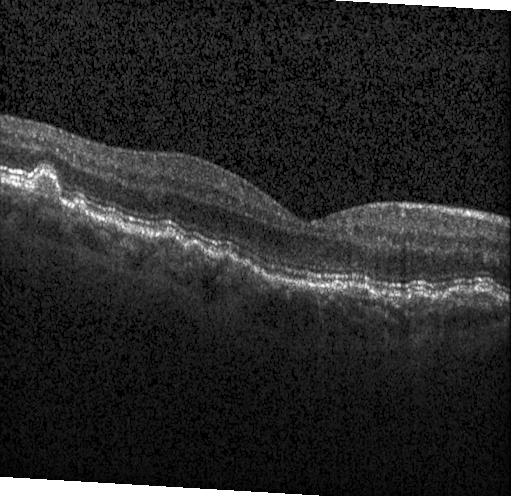
Diagnosis: sub-RPE drusenoid deposits.